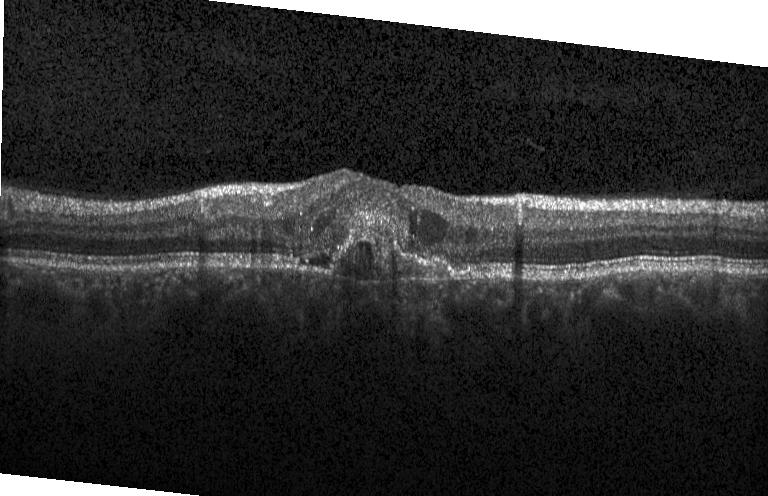 Acquired on a Heidelberg Spectralis · OCT B-scan. Assessment: a choroidal neovascular membrane.